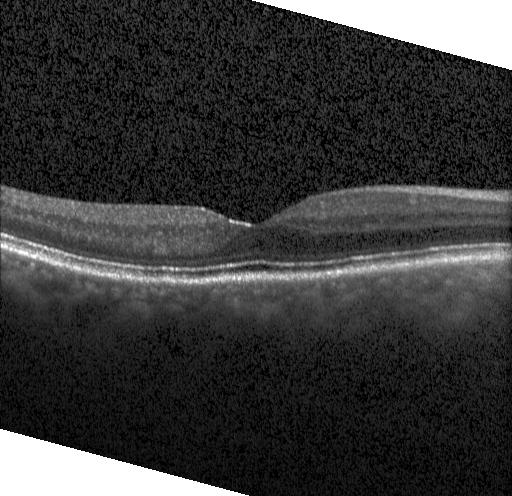
Impression: neither CNV, DME, nor drusen.